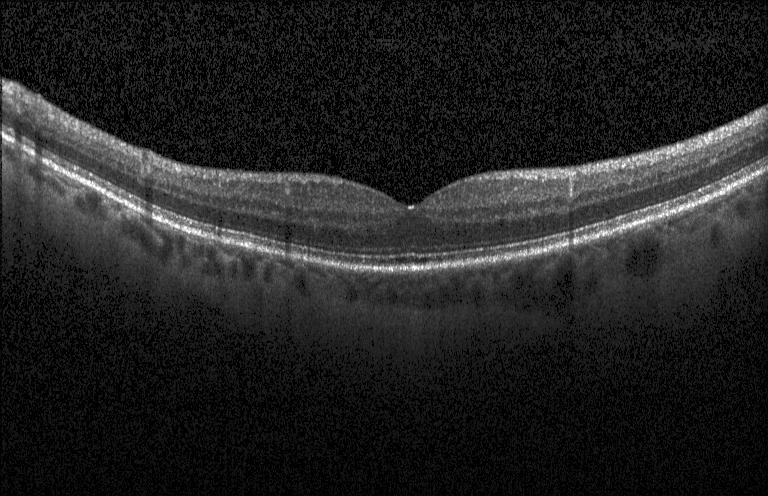

Retinal OCT B-scan
This B-scan demonstrates neither choroidal neovascularization, diabetic macular edema, nor drusen.